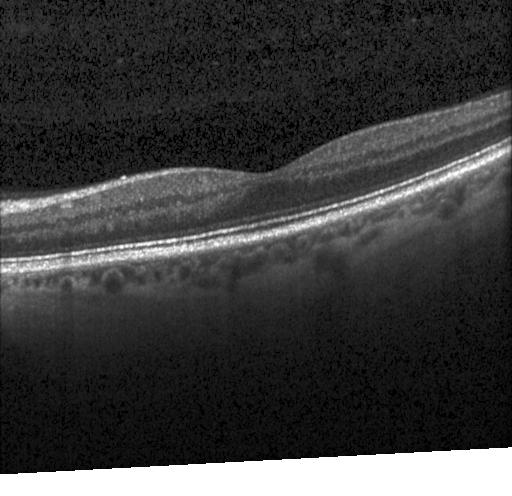

Spectral-domain optical coherence tomography; OCT B-scan. OCT finding: no CNV, no DME, and no drusen.